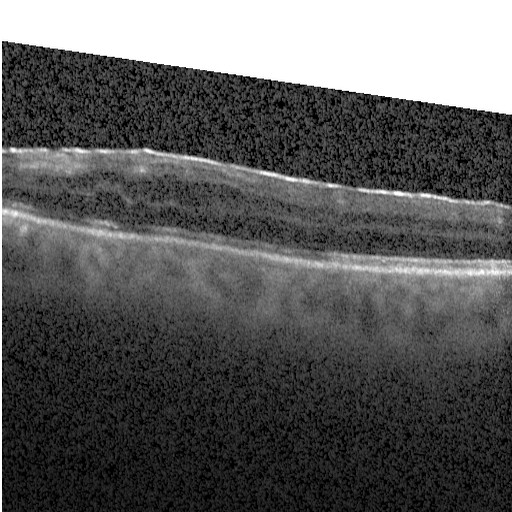
OCT B-scan. Diagnosis: DME.